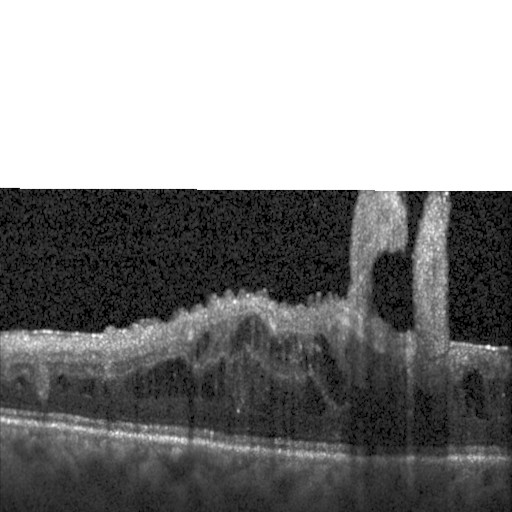

Spectral-domain OCT. Retinal OCT B-scan. Fovea-centered. Impression: DME.